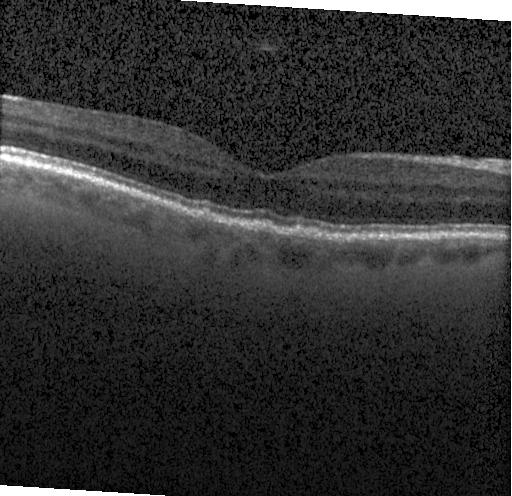
Retinal OCT cross-section — Macular OCT: sub-RPE drusenoid deposits.